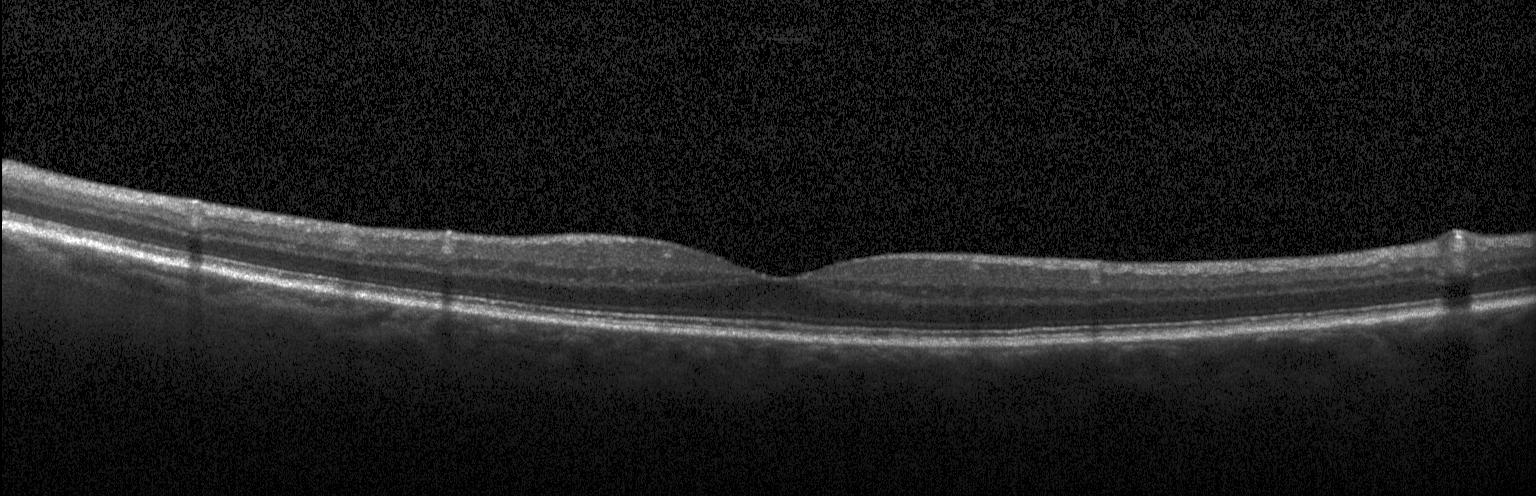

Retinal OCT B-scan.
The scan shows no choroidal neovascularization, no diabetic macular edema, and no drusen.